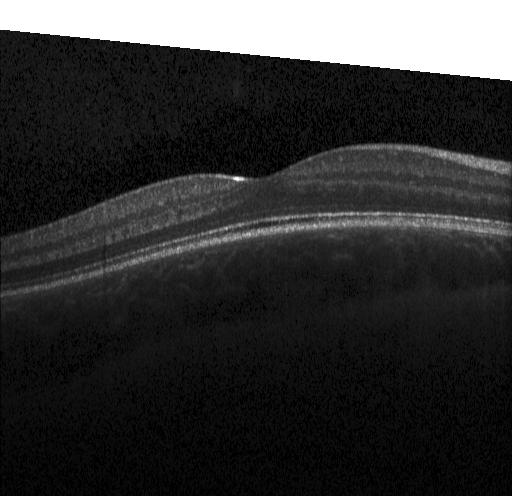

Macular scan · spectral-domain OCT · retinal OCT cross-section — Diagnosis: no CNV, DME, or drusen.